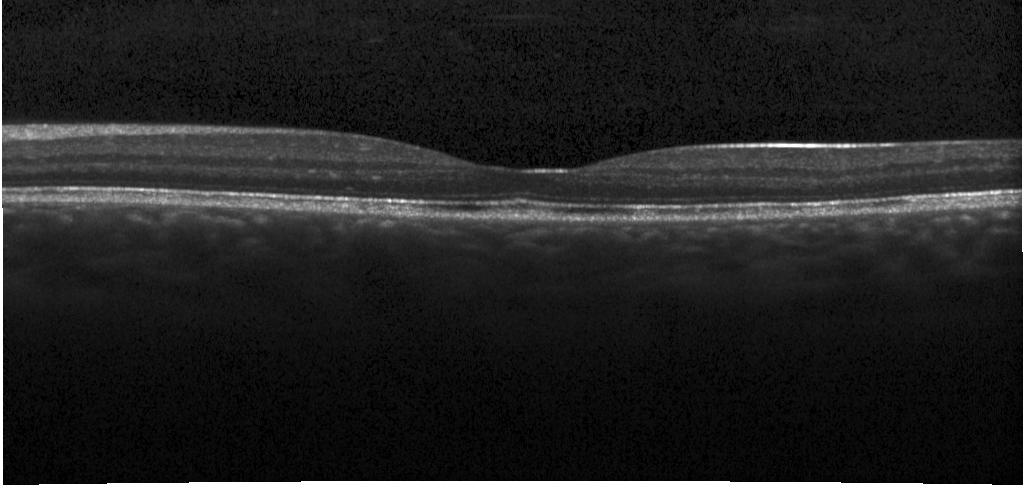
Retinal OCT B-scan.
Macular OCT: no CNV, DME, or drusen.